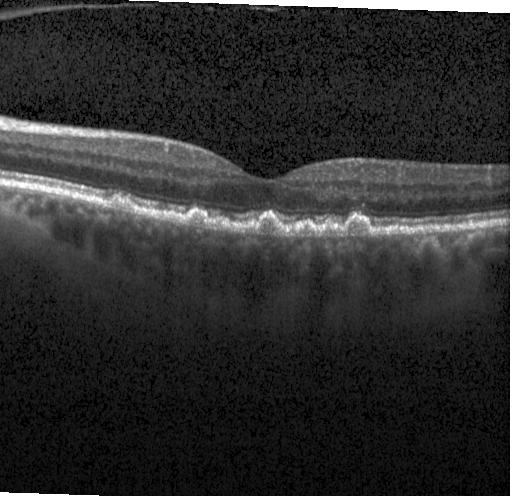
Horizontal scan through the fovea. Retinal OCT B-scan. Diagnosis: sub-RPE drusenoid deposits.